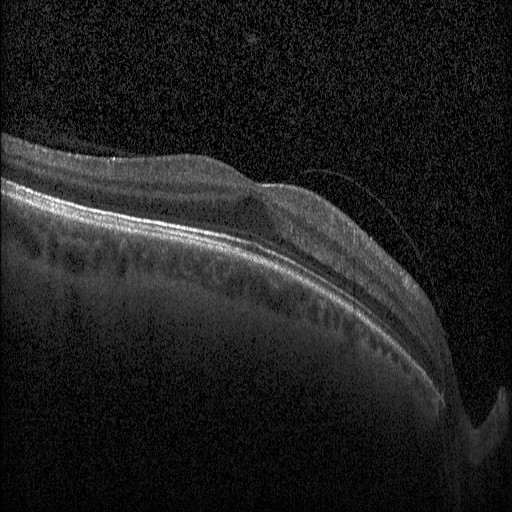 Horizontal scan through the fovea, Heidelberg Spectralis OCT system, retinal OCT B-scan.
The scan shows diabetic macular edema.